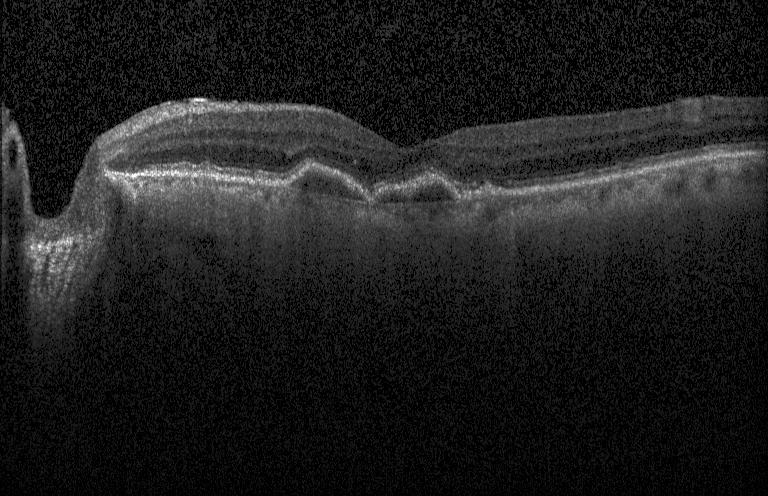

Impression: a choroidal neovascular membrane.